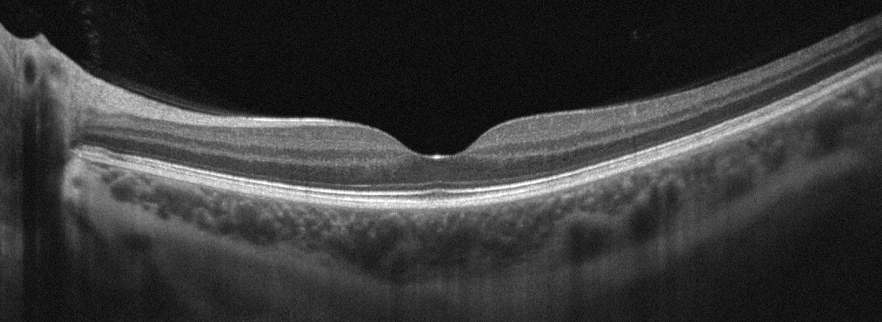
Retinal OCT B-scan. Oculus sinister
Finding: no AMD, DME, ERM, RAO, RVO, or VID.